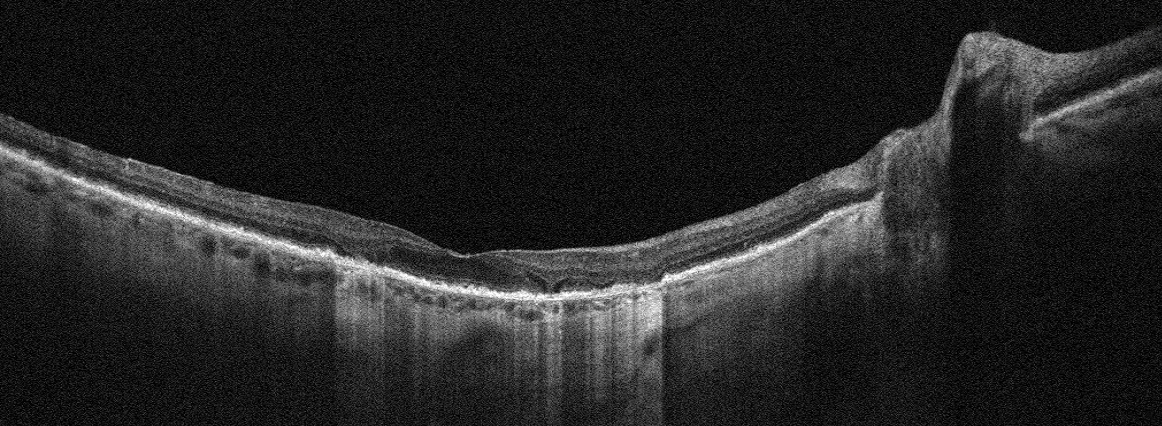
OCT B-scan · acquired on an Optovue Avanti RTVue XR · oculus dexter · fovea-centered. OCT finding: age-related macular degeneration.